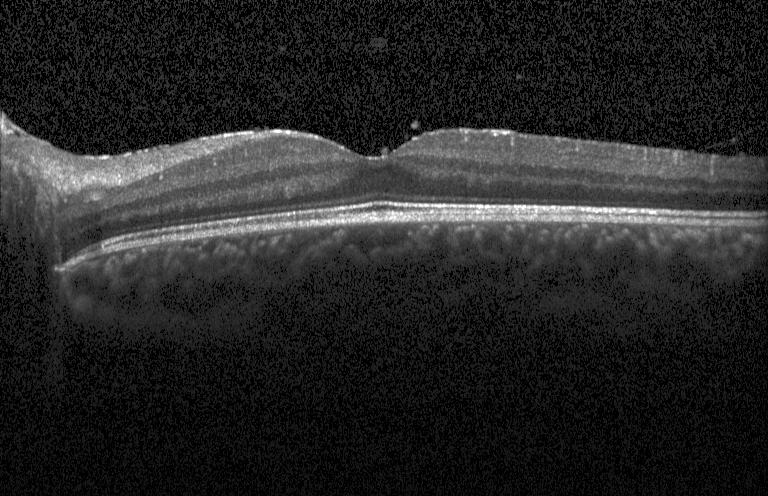
OCT finding: neither choroidal neovascularization, diabetic macular edema, nor drusen.